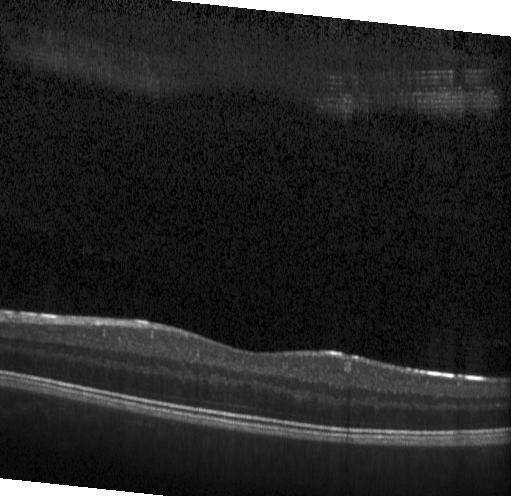
Through the macula. Retinal OCT B-scan. The scan shows no evidence of choroidal neovascularization, diabetic macular edema, or drusen.